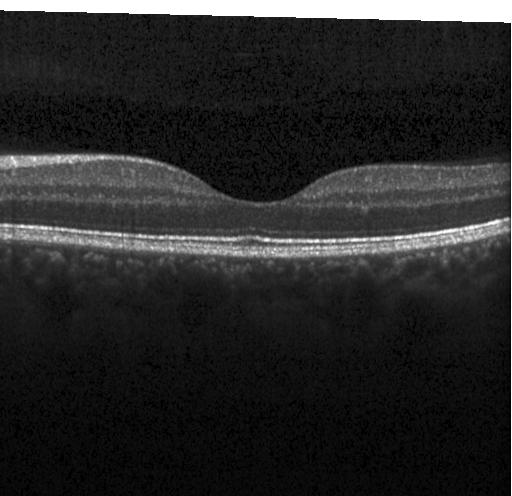 Instrument: Heidelberg Spectralis, spectral-domain OCT, optical coherence tomography scan.
No CNV, no DME, and no drusen.